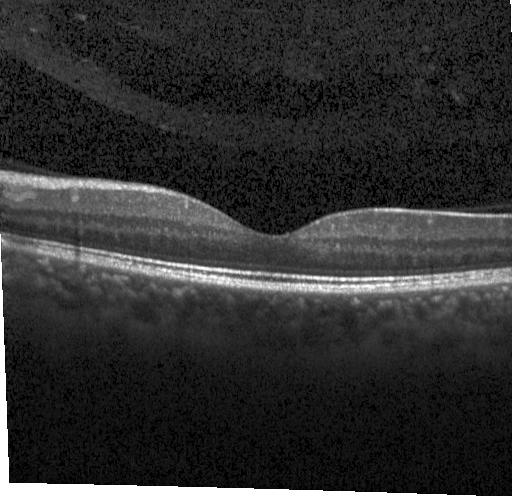

Spectral-domain OCT, centered on the fovea, optical coherence tomography B-scan
This B-scan demonstrates no choroidal neovascularization, diabetic macular edema, or drusen.